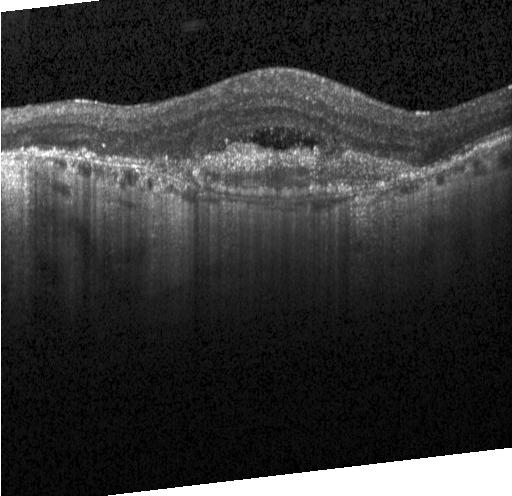

Spectral-domain optical coherence tomography · OCT B-scan · through the macula · instrument: Heidelberg Spectralis
Macular OCT: a choroidal neovascular membrane.